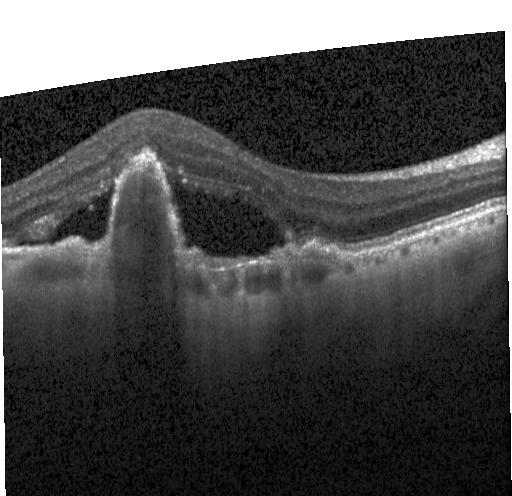

OCT line scan. SD-OCT. Macular scan.
Macular OCT: a choroidal neovascular membrane.